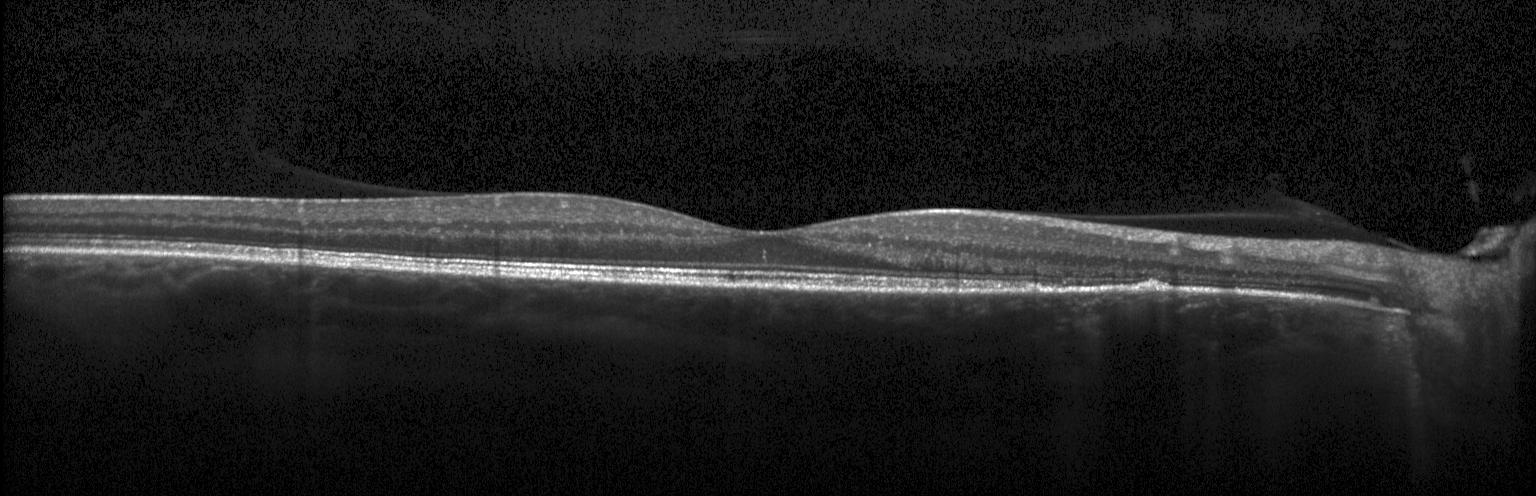 Heidelberg Spectralis OCT system. Spectral-domain OCT. OCT B-scan. Centered on the fovea
This B-scan demonstrates neither choroidal neovascularization, diabetic macular edema, nor drusen.